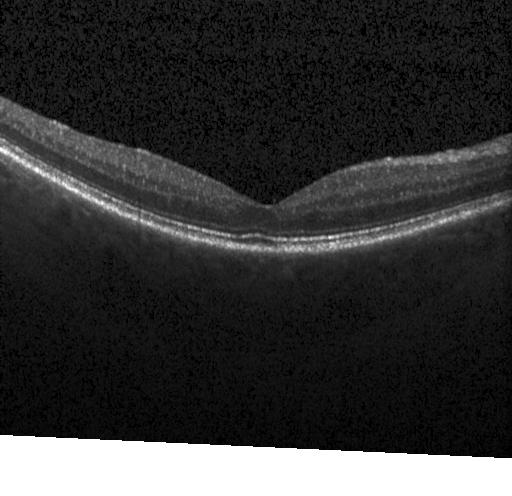
OCT line scan
Diagnosis: no evidence of choroidal neovascularization, diabetic macular edema, or drusen.